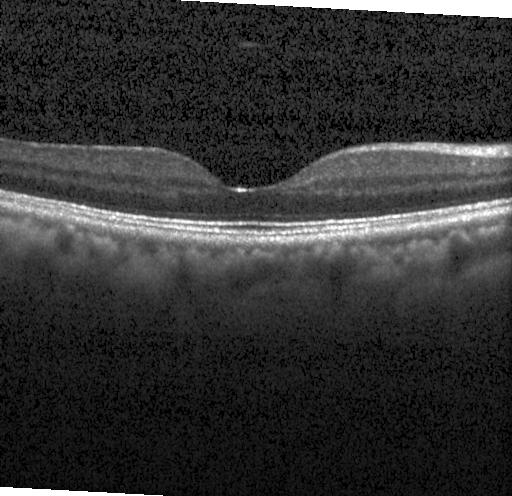
Heidelberg Spectralis, retinal OCT cross-section — Diagnosis: no choroidal neovascularization, no diabetic macular edema, and no drusen.